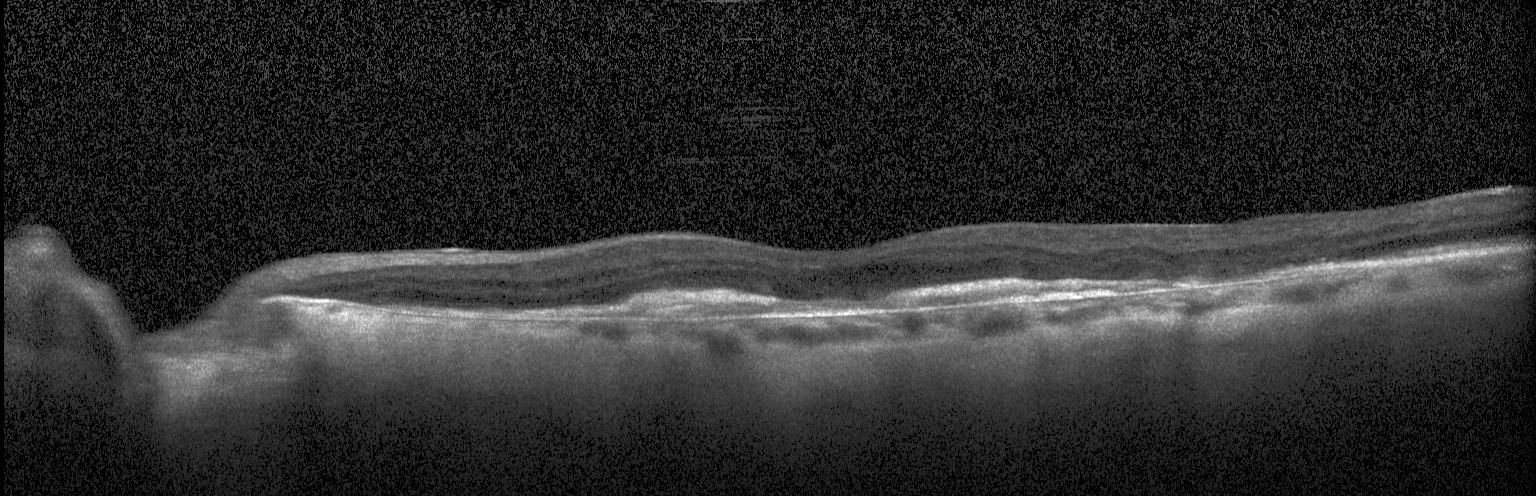 SD-OCT. OCT B-scan.
This B-scan demonstrates choroidal neovascularization (CNV).